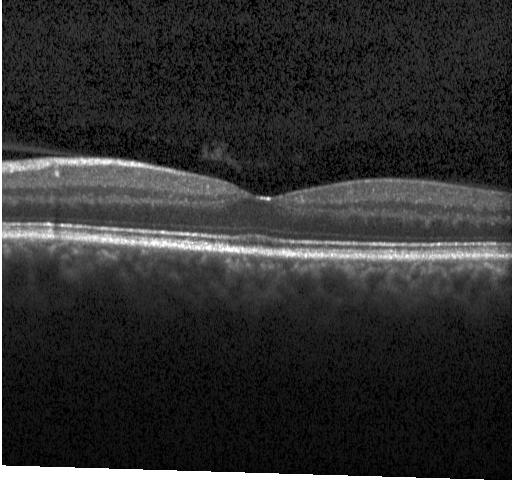

Retinal OCT B-scan. Spectral-domain optical coherence tomography. Centered on the fovea. Instrument: Heidelberg Spectralis
Macular OCT: no evidence of CNV, DME, or drusen.